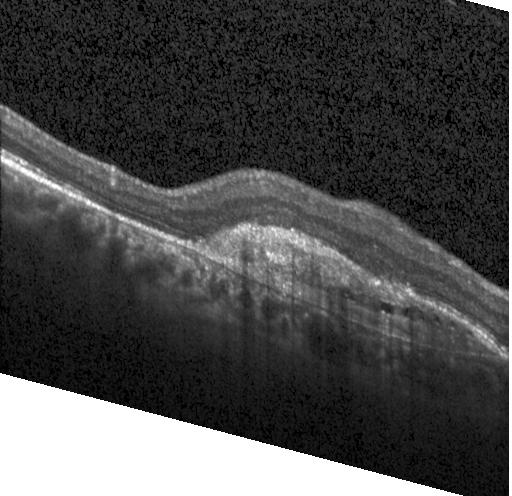 Optical coherence tomography scan
This B-scan demonstrates a choroidal neovascular membrane.